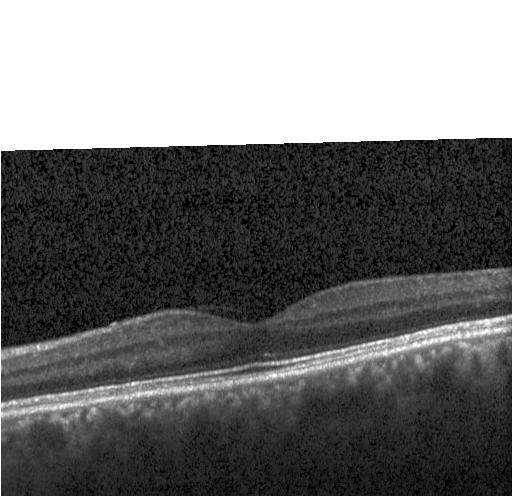 Finding: no choroidal neovascularization, no diabetic macular edema, and no drusen.